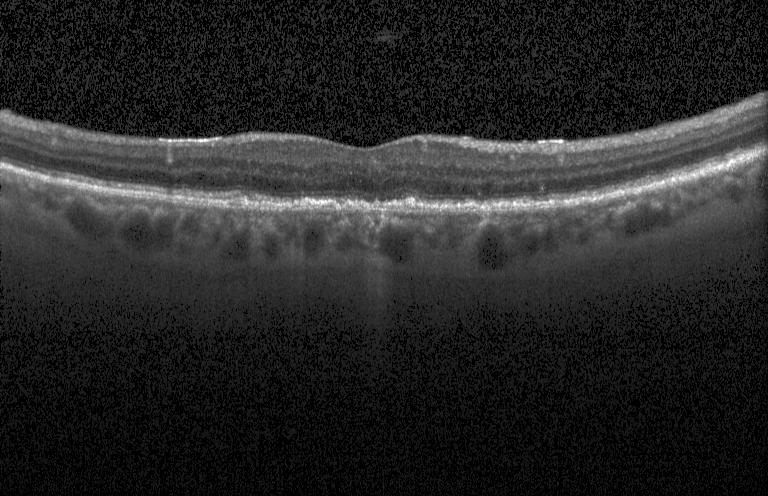 OCT B-scan.
The scan shows CNV.